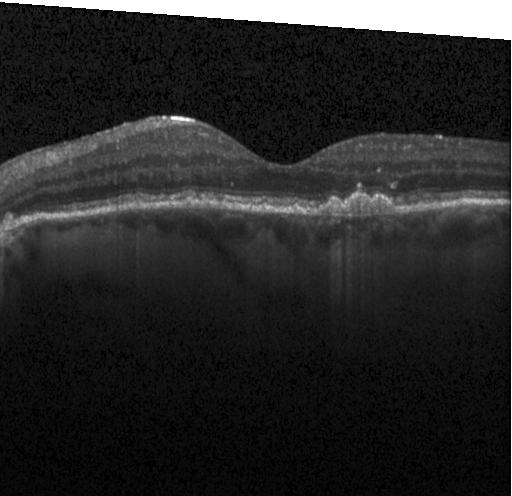 The scan shows drusen.